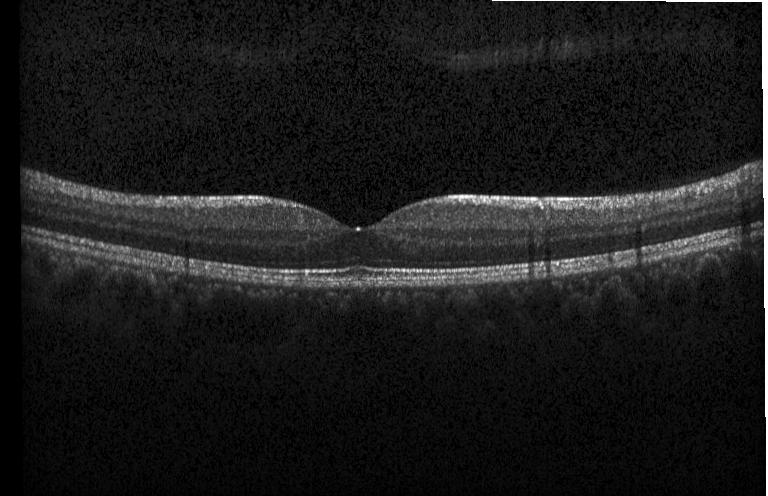 OCT line scan · spectral-domain optical coherence tomography
Diagnosis: no CNV, no DME, and no drusen.